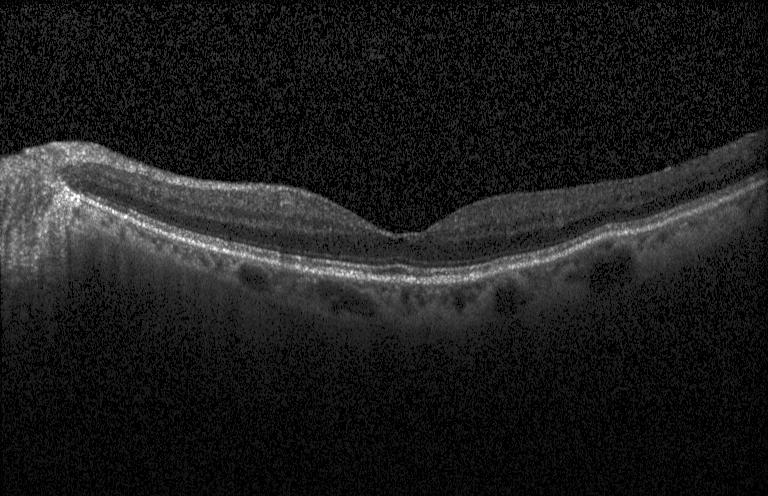 Optical coherence tomography B-scan. Centered on the fovea. Heidelberg Spectralis OCT system.
OCT finding: no CNV, DME, or drusen.